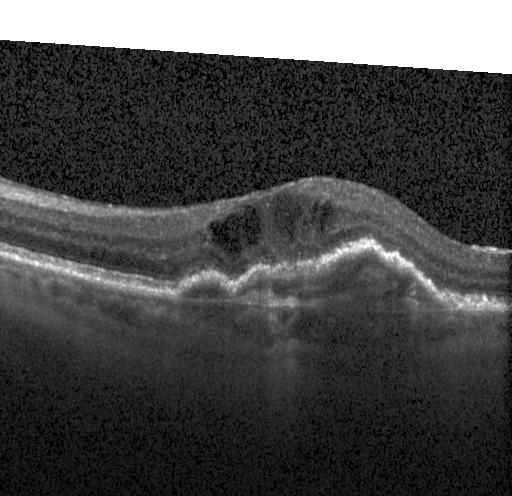 Macular OCT demonstrating choroidal neovascularization (CNV).